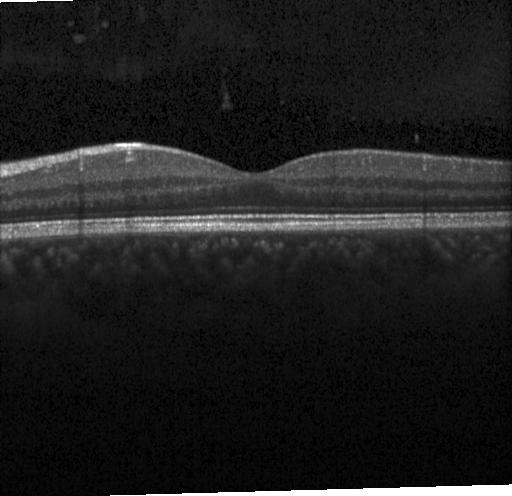
Fovea-centered. Instrument: Heidelberg Spectralis. Retinal OCT B-scan. Spectral-domain optical coherence tomography.
The scan shows no choroidal neovascularization, diabetic macular edema, or drusen.